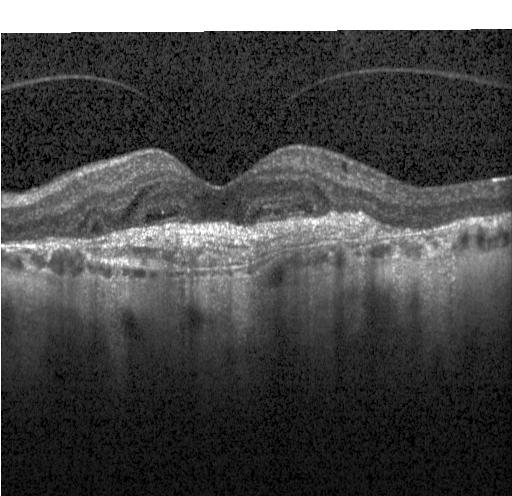

Acquired on a Heidelberg Spectralis; horizontal scan through the fovea; optical coherence tomography B-scan; spectral-domain optical coherence tomography. The scan shows a choroidal neovascular membrane.